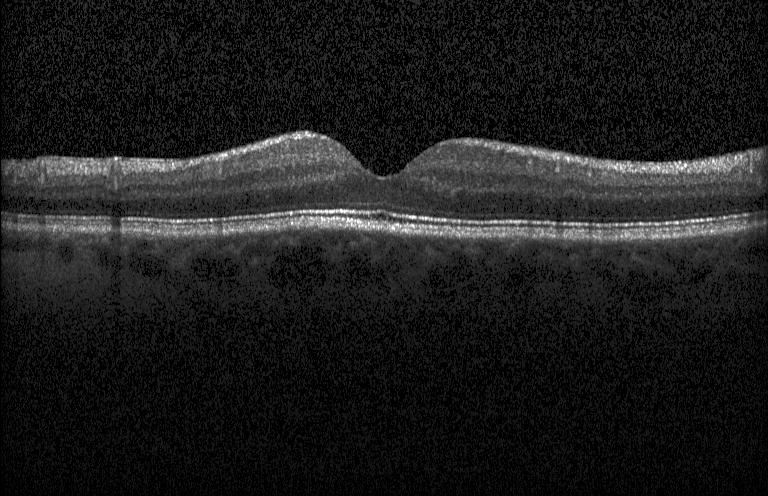
OCT finding: no evidence of CNV, DME, or drusen.